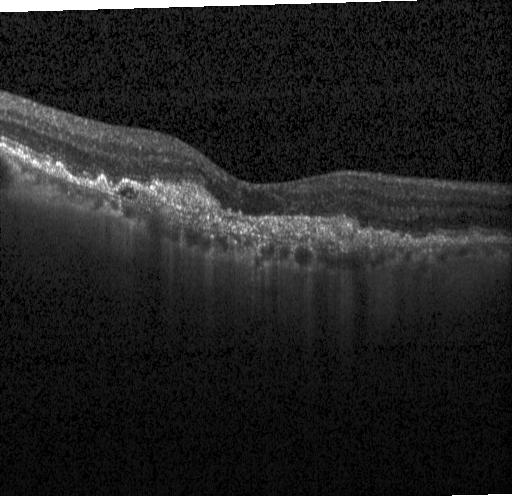

OCT line scan. Spectral-domain optical coherence tomography
Dx: choroidal neovascularization.